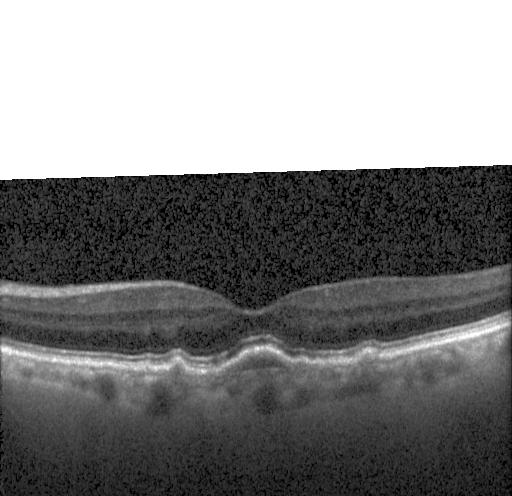
Diagnosis: choroidal neovascularization (CNV).